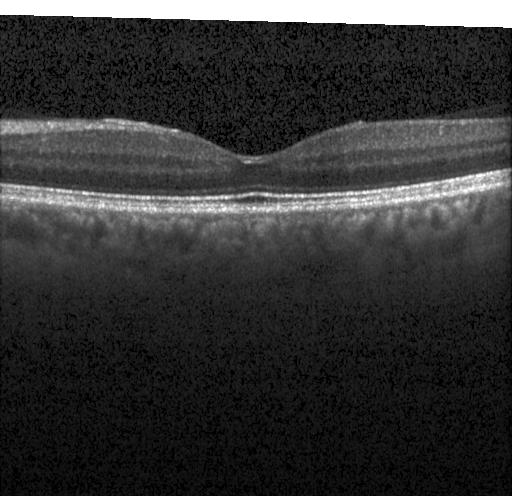

Instrument: Heidelberg Spectralis; through the macula; SD-OCT; retinal OCT B-scan
Assessment: no evidence of choroidal neovascularization, diabetic macular edema, or drusen.